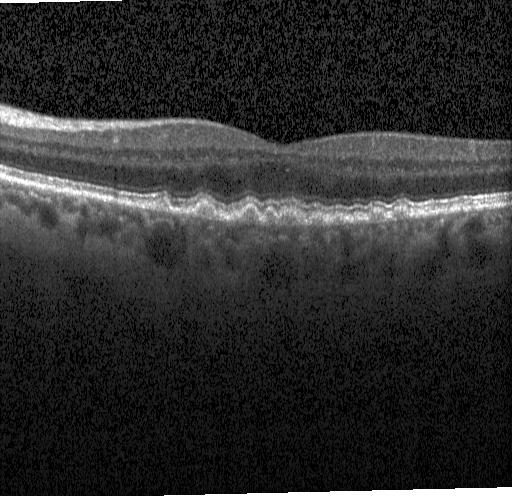
Fovea-centered, Heidelberg Spectralis, OCT B-scan. Diagnosis: sub-RPE drusenoid deposits.